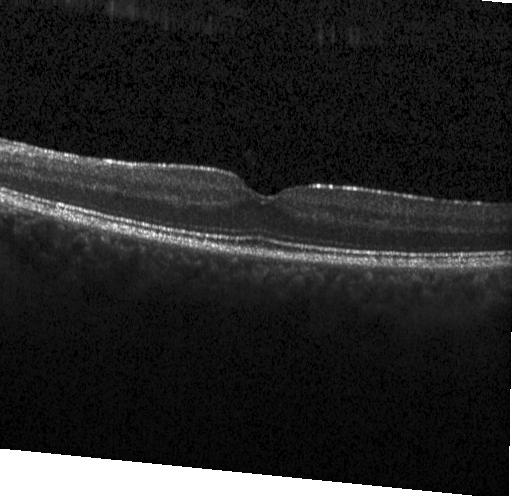 OCT line scan, Heidelberg Spectralis — This B-scan demonstrates no CNV, DME, or drusen.